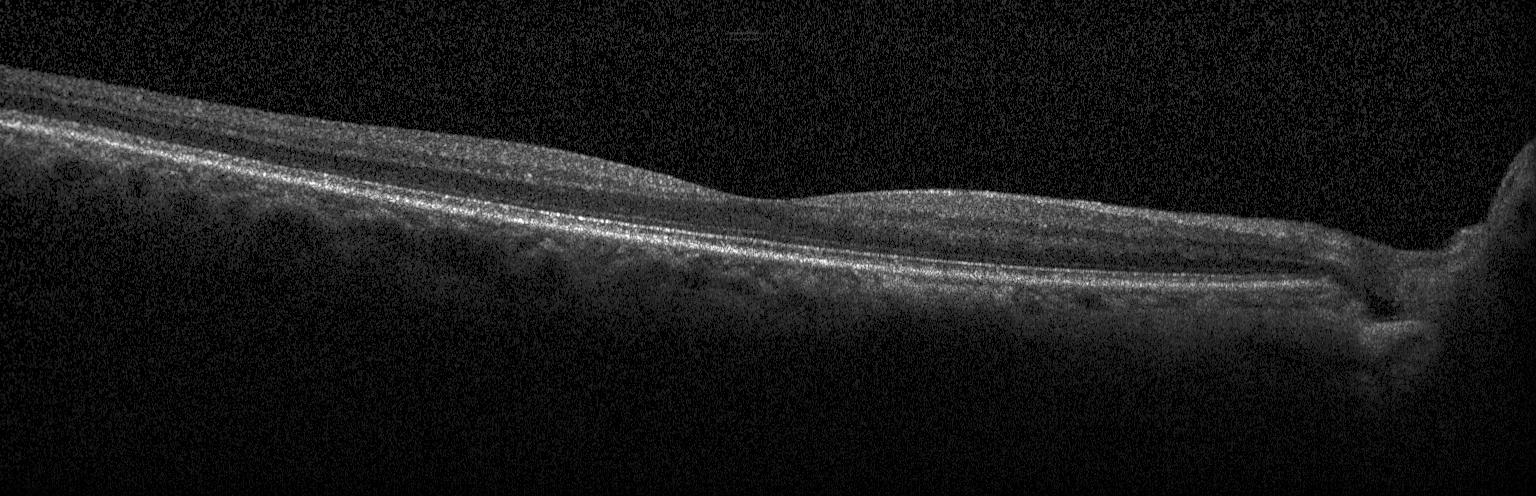
Spectral-domain OCT. OCT B-scan. Diagnosis: no evidence of choroidal neovascularization, diabetic macular edema, or drusen.